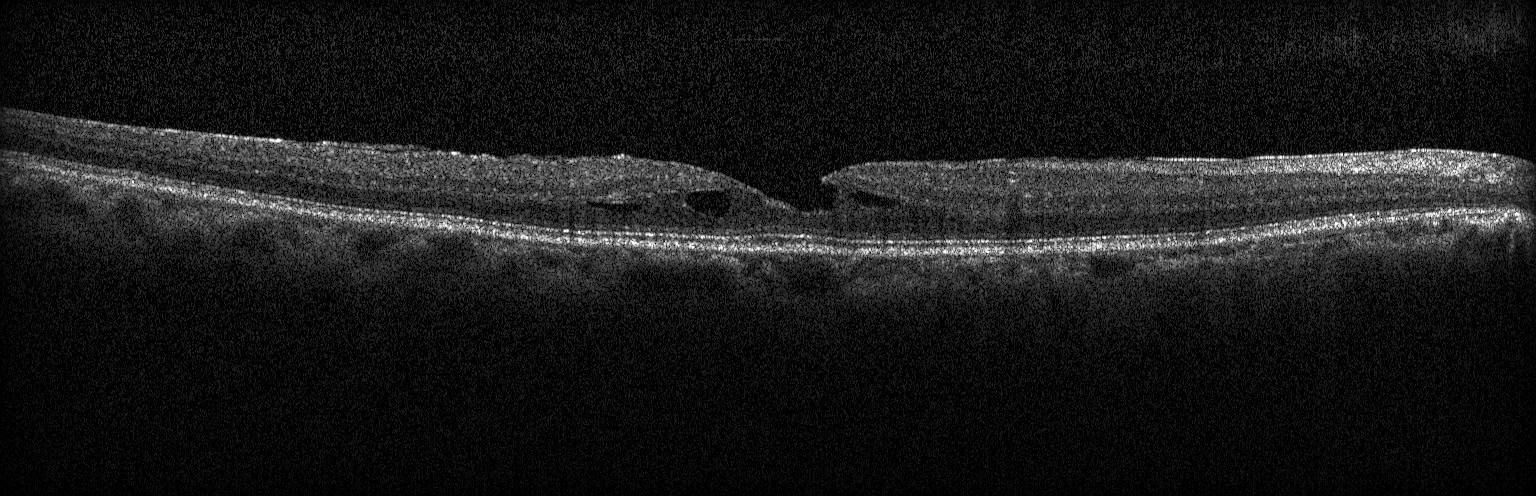
Impression: DME.